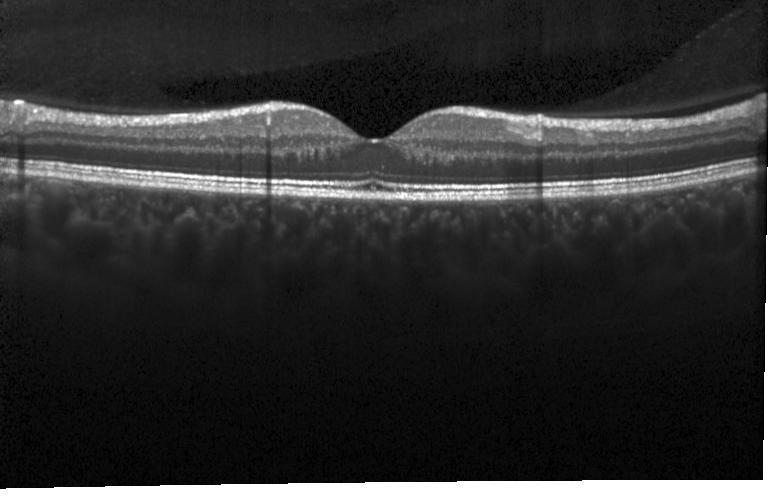

Macular scan · SD-OCT · optical coherence tomography B-scan.
OCT finding: neither choroidal neovascularization, diabetic macular edema, nor drusen.